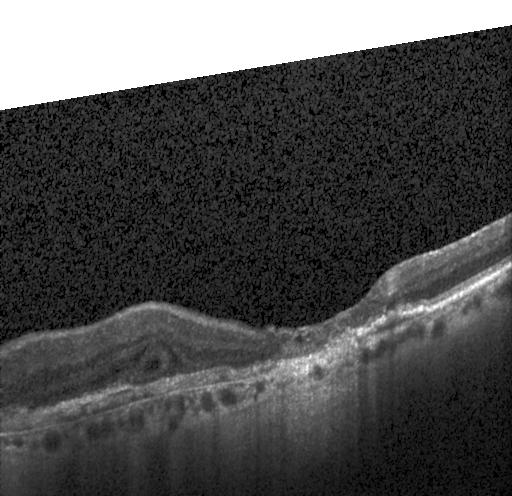
Retinal OCT cross-section. Heidelberg Spectralis OCT system.
Diagnosis: a choroidal neovascular membrane.